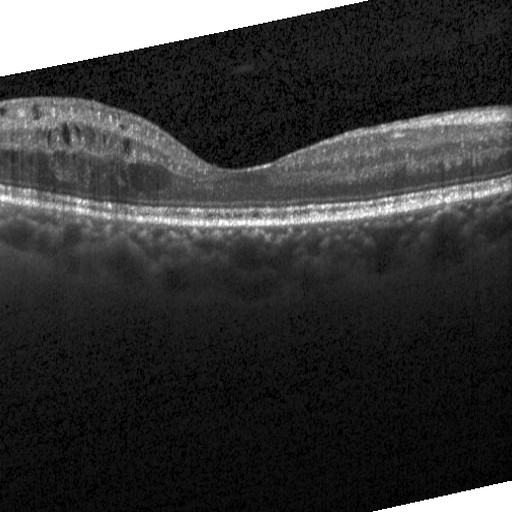 Spectral-domain optical coherence tomography. Optical coherence tomography scan — Diagnosis: diabetic macular edema (DME).